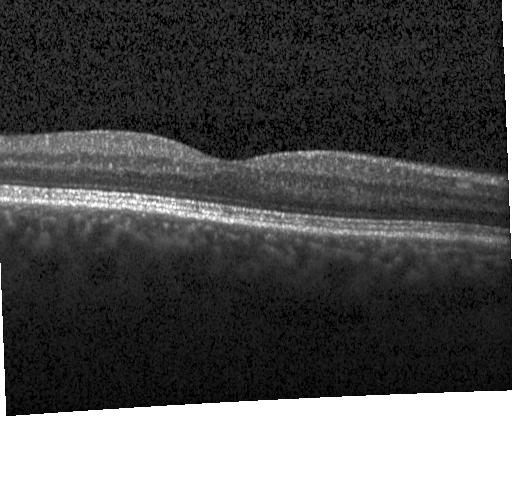
OCT finding: no choroidal neovascularization, diabetic macular edema, or drusen.